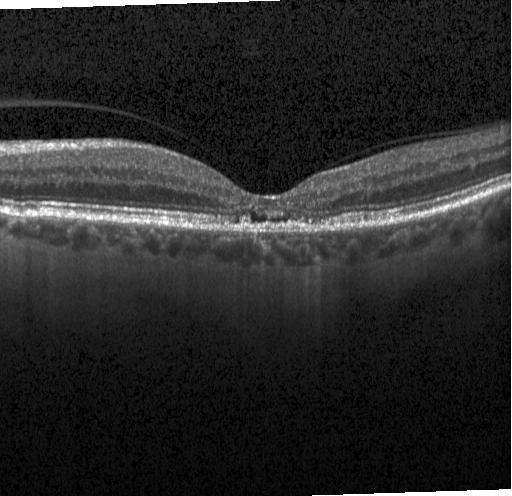
Spectral-domain optical coherence tomography, Heidelberg Spectralis, optical coherence tomography B-scan
The scan shows choroidal neovascularization (CNV).